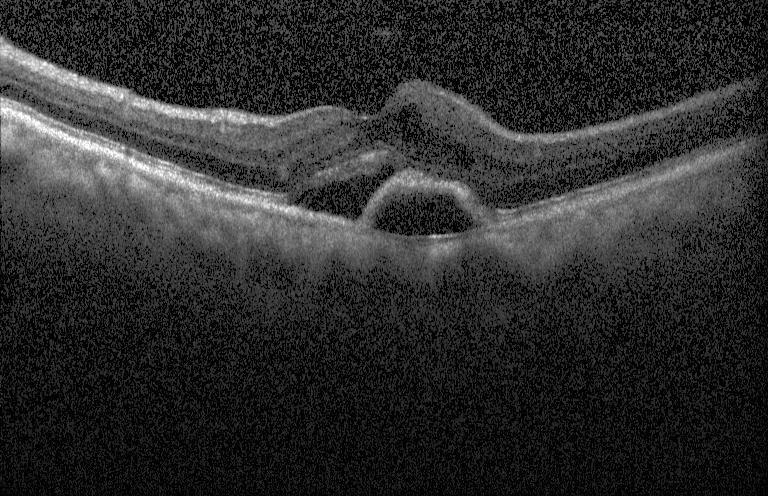
Retinal OCT B-scan. Diagnosis: a choroidal neovascular membrane.